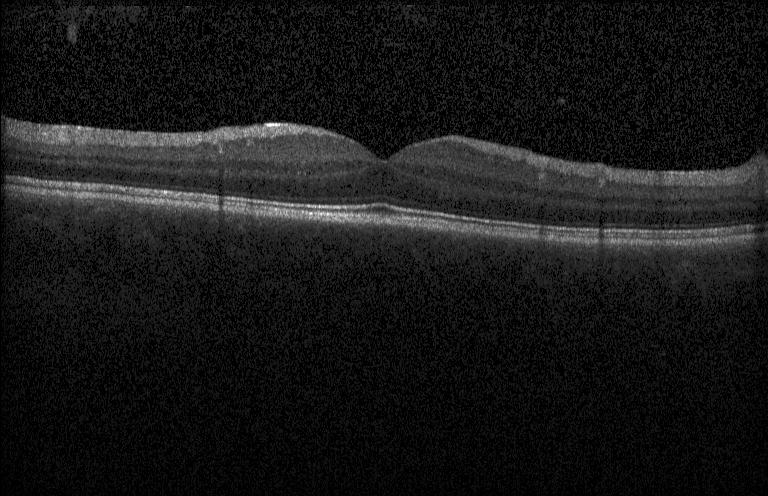 Optical coherence tomography B-scan.
Finding: no evidence of choroidal neovascularization, diabetic macular edema, or drusen.